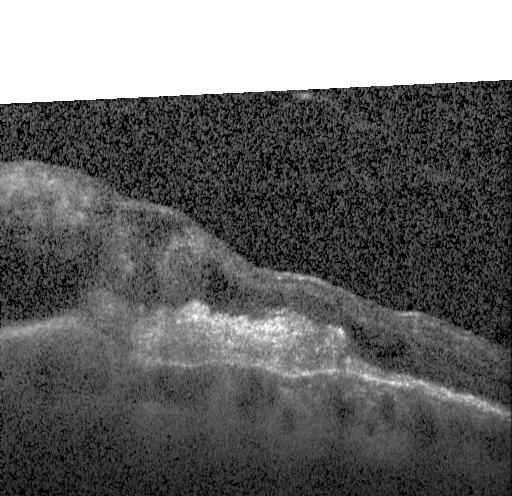 Optical coherence tomography scan. Assessment: choroidal neovascularization.